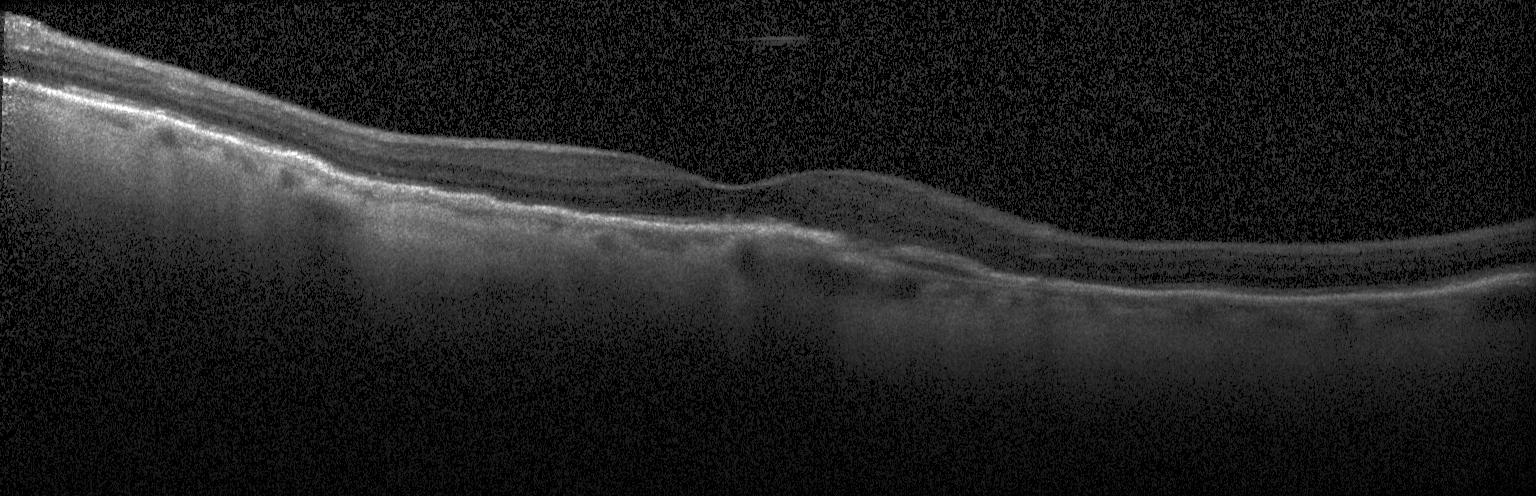 OCT finding: a choroidal neovascular membrane.